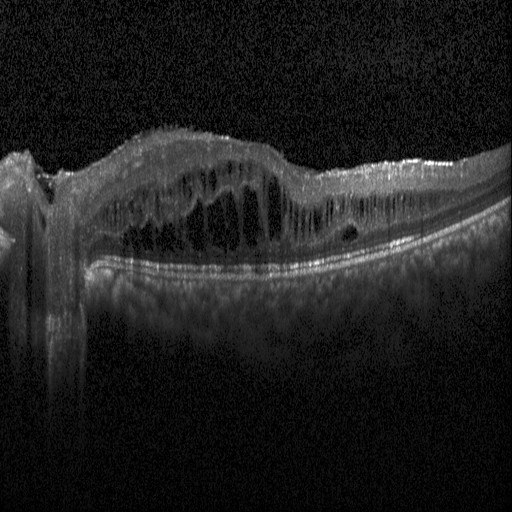 Through the macula · retinal OCT B-scan — Impression: DME.